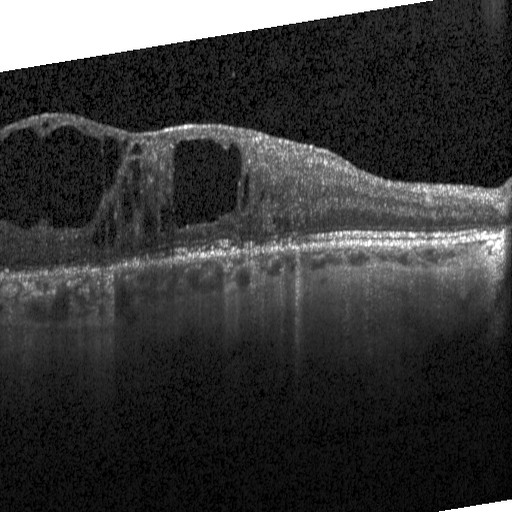 Spectral-domain optical coherence tomography. Centered on the fovea. OCT line scan
Macular OCT: diabetic macular edema (DME).